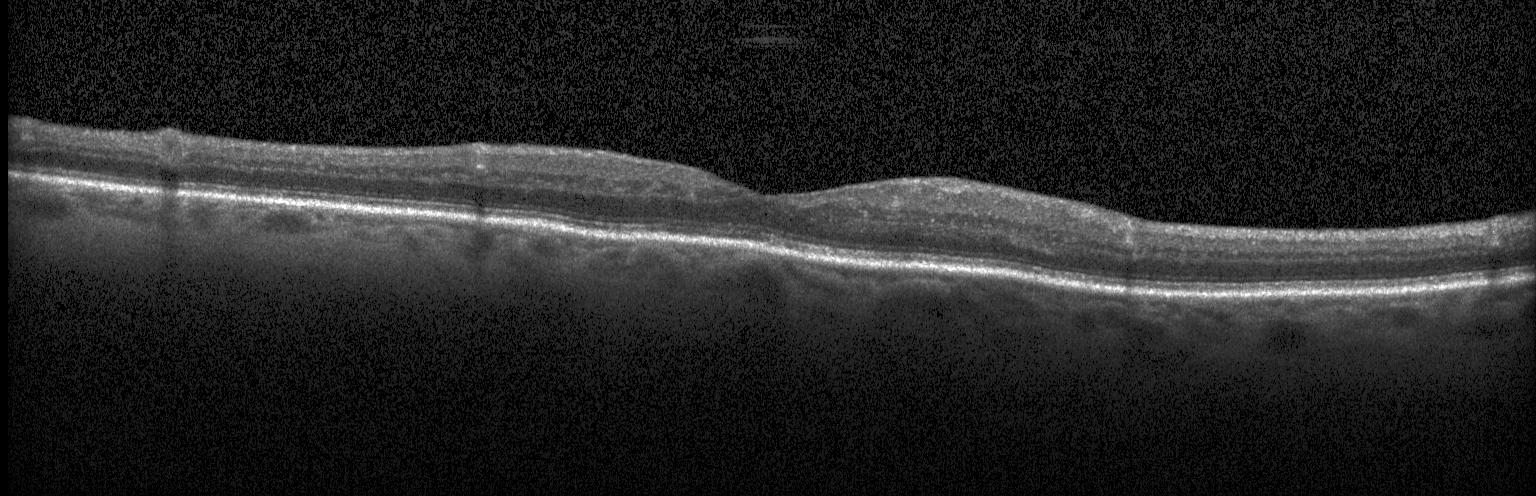
Assessment: neither CNV, DME, nor drusen.